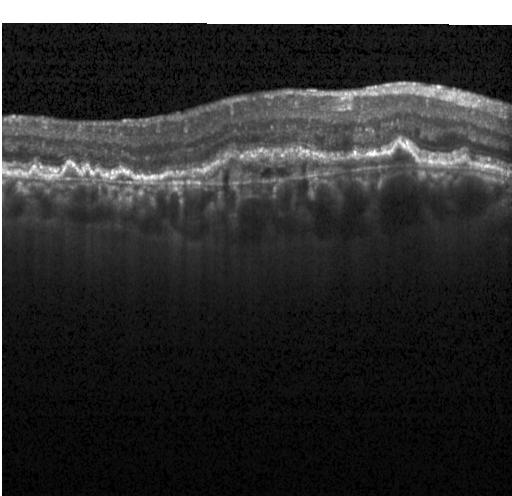 Macular OCT: choroidal neovascularization.